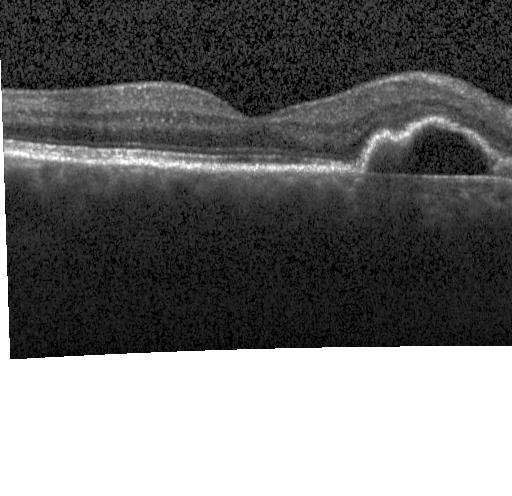 Optical coherence tomography B-scan, spectral-domain OCT, centered on the fovea, acquired on a Heidelberg Spectralis. Impression: CNV.